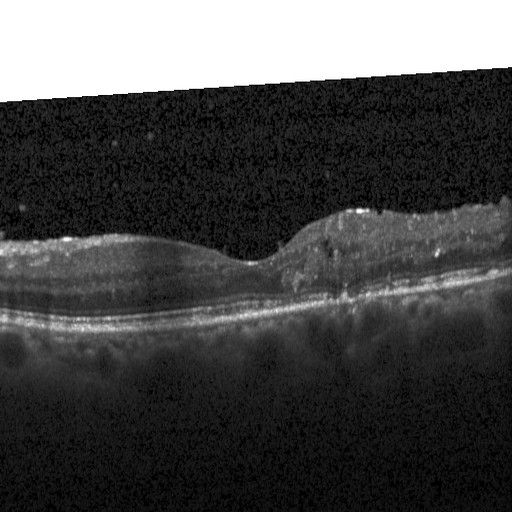

Through the macula, Heidelberg Spectralis OCT system, OCT line scan — The scan shows DME.